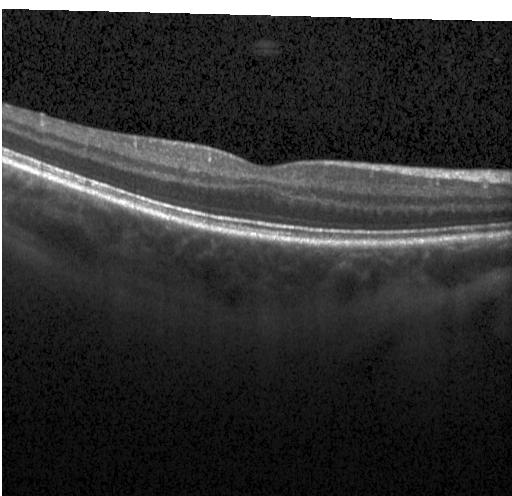

SD-OCT, optical coherence tomography B-scan — Assessment: no evidence of choroidal neovascularization, diabetic macular edema, or drusen.